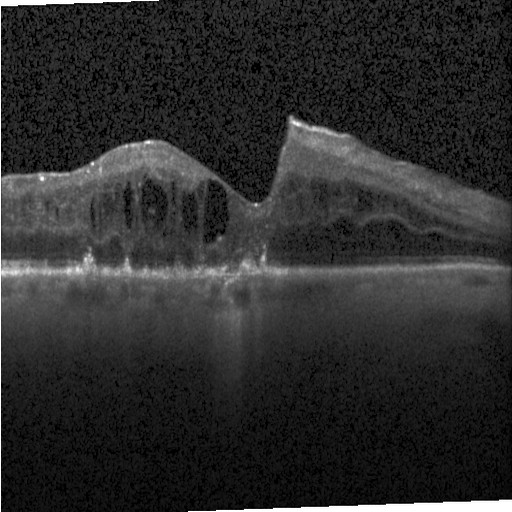 OCT B-scan showing DME.